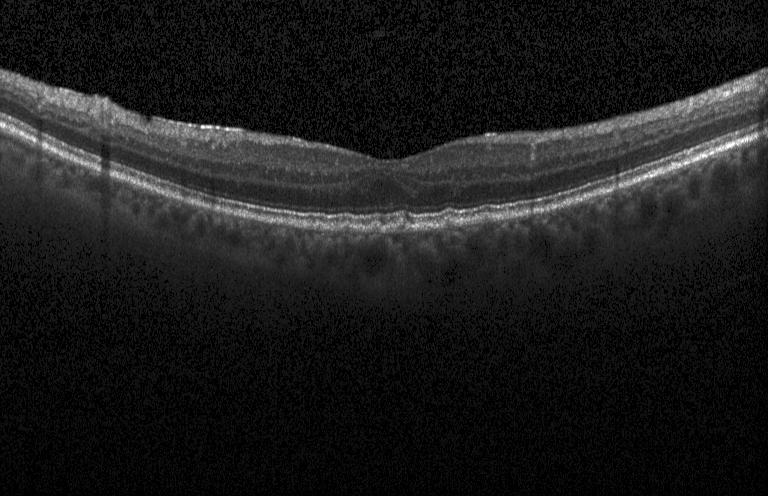
Heidelberg Spectralis OCT system, through the macula, optical coherence tomography B-scan, spectral-domain optical coherence tomography — Dx: drusen.